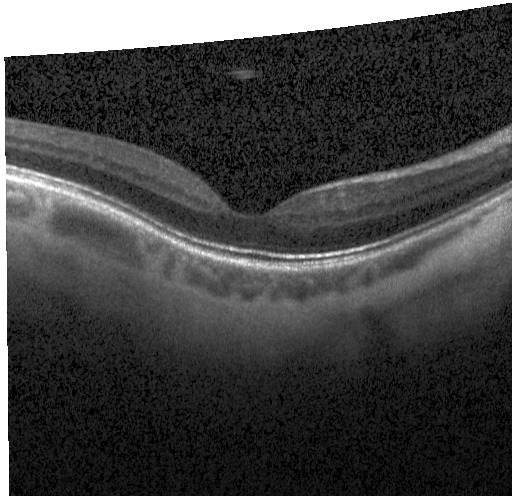

Retinal OCT cross-section
Finding: neither choroidal neovascularization, diabetic macular edema, nor drusen.